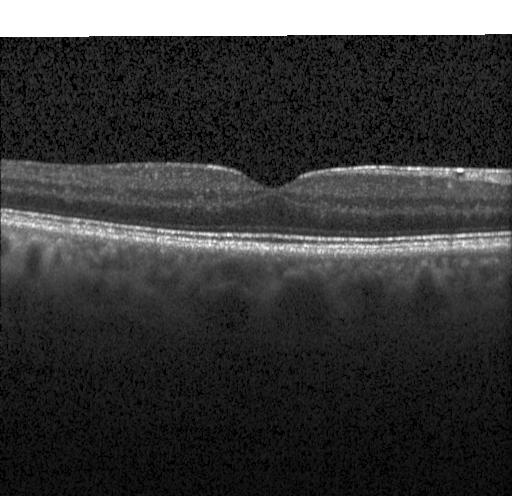

SD-OCT. OCT line scan
Macular OCT: neither choroidal neovascularization, diabetic macular edema, nor drusen.